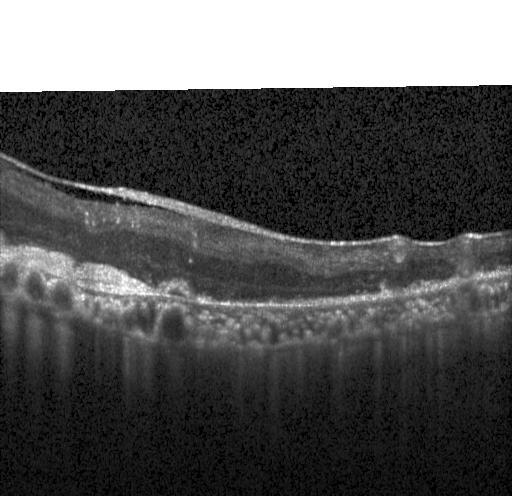

Finding: a choroidal neovascular membrane.